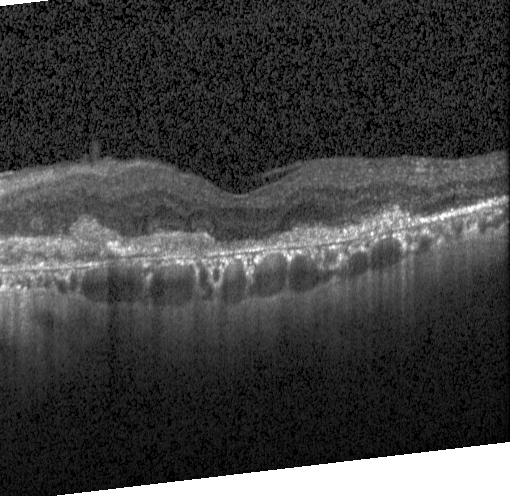
Retinal OCT cross-section, acquired on a Heidelberg Spectralis, spectral-domain optical coherence tomography. Finding: a choroidal neovascular membrane.